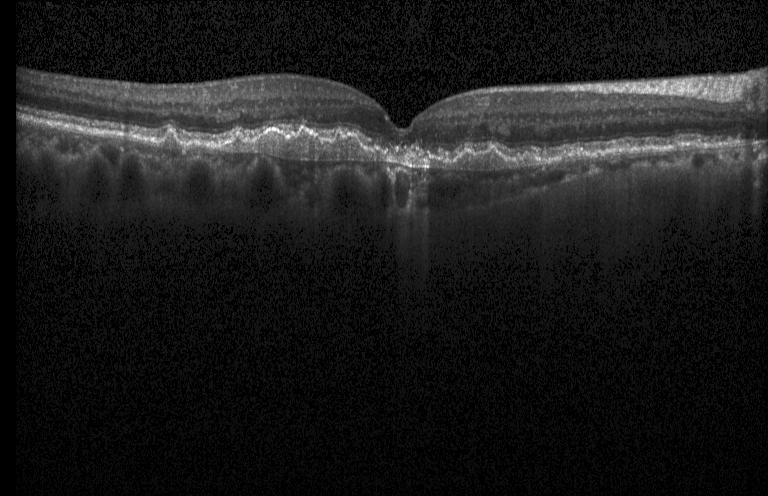

Instrument: Heidelberg Spectralis · through the macula · retinal OCT cross-section — Assessment: choroidal neovascularization (CNV).